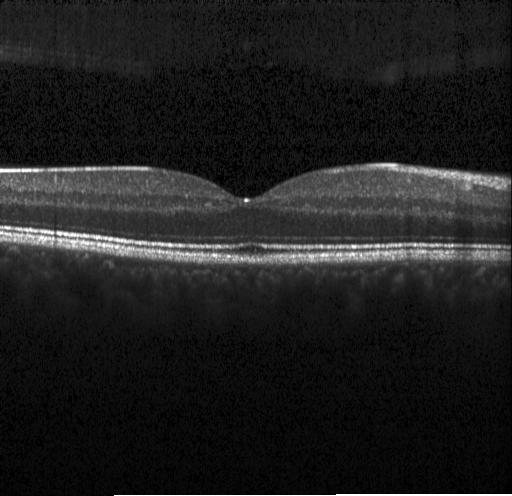

OCT line scan. Heidelberg Spectralis OCT system. Spectral-domain OCT. Macular scan
No choroidal neovascularization, no diabetic macular edema, and no drusen.